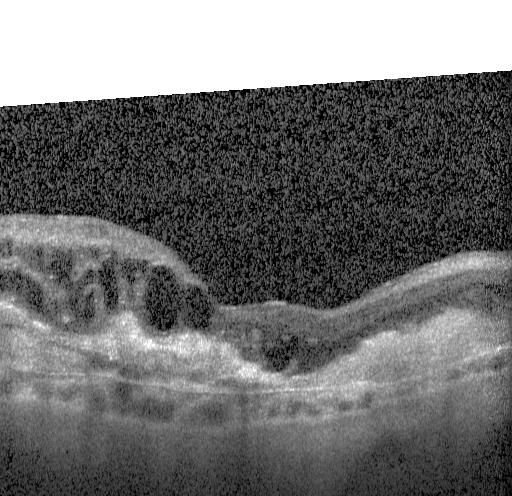 Impression: a choroidal neovascular membrane.